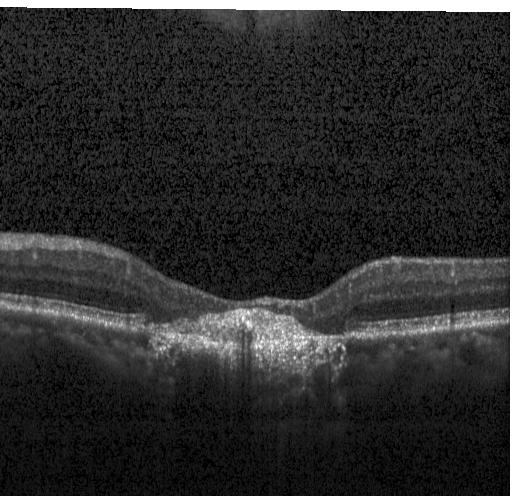

OCT finding: a choroidal neovascular membrane.